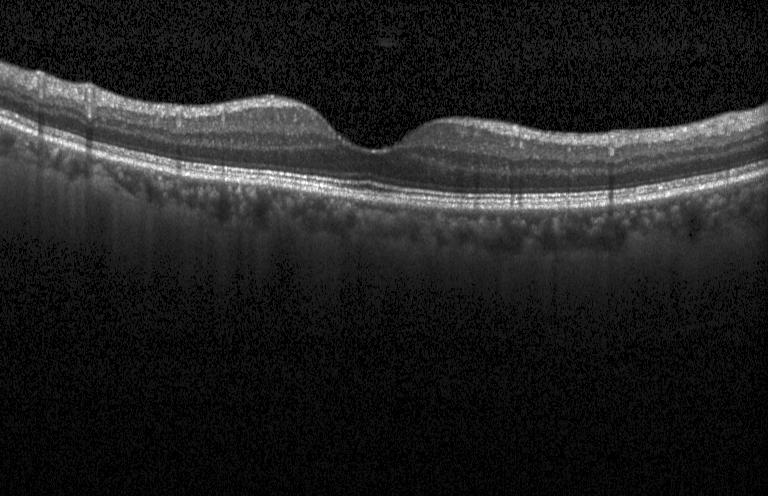

OCT finding: no evidence of choroidal neovascularization, diabetic macular edema, or drusen.